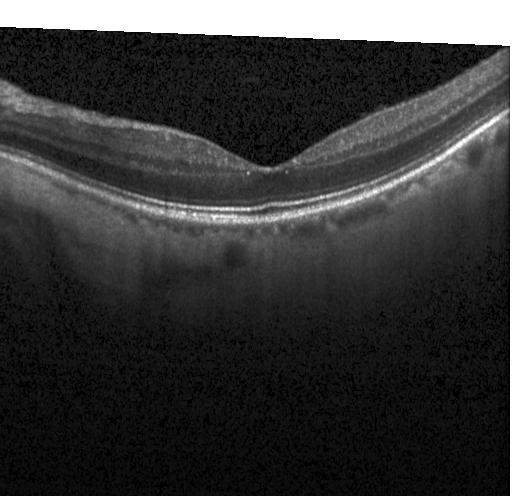
Macular OCT: no evidence of choroidal neovascularization, diabetic macular edema, or drusen.